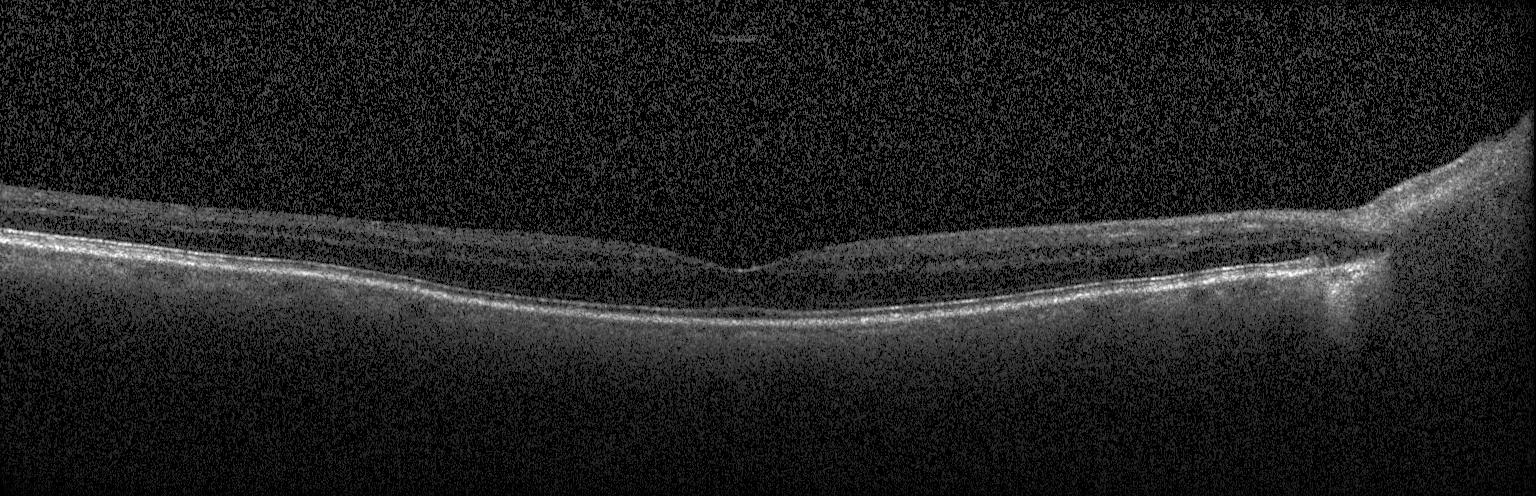 Acquired on a Heidelberg Spectralis · optical coherence tomography B-scan · centered on the fovea.
Impression: no choroidal neovascularization, diabetic macular edema, or drusen.